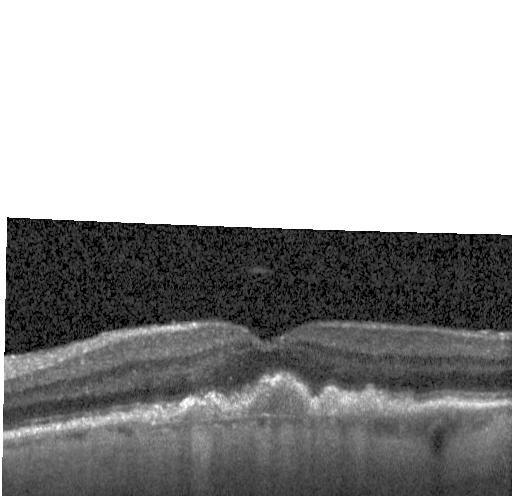

Heidelberg Spectralis OCT system · macular scan · optical coherence tomography scan. This B-scan demonstrates a choroidal neovascular membrane.